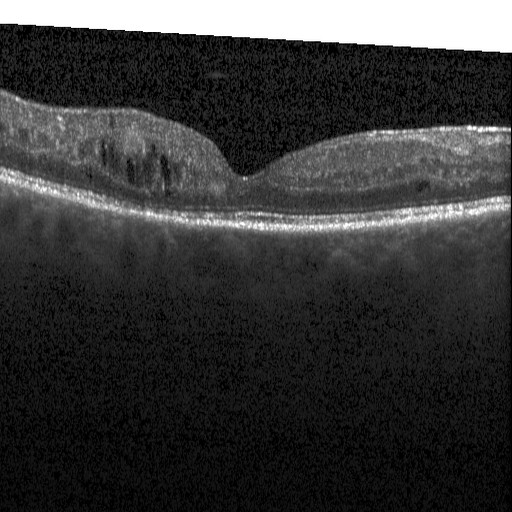 OCT B-scan · centered on the fovea · instrument: Heidelberg Spectralis. Dx: DME.